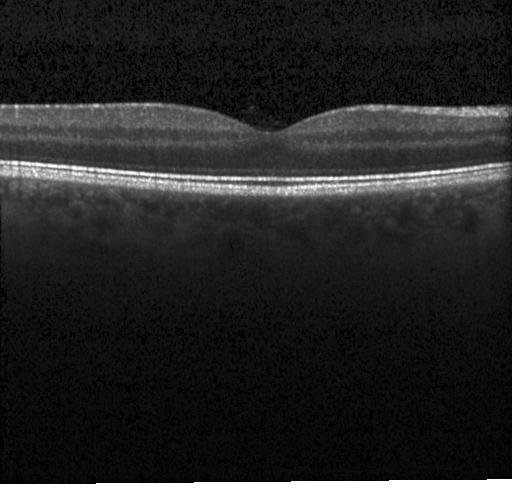 Optical coherence tomography B-scan.
Assessment: no CNV, no DME, and no drusen.